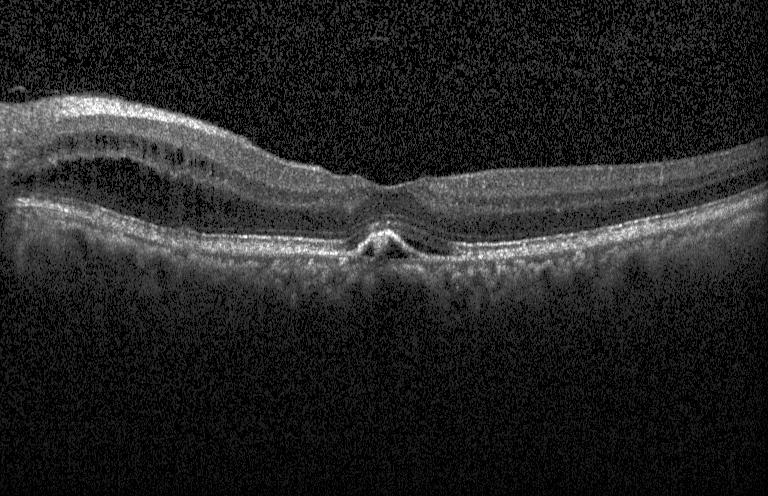 Finding: a choroidal neovascular membrane.